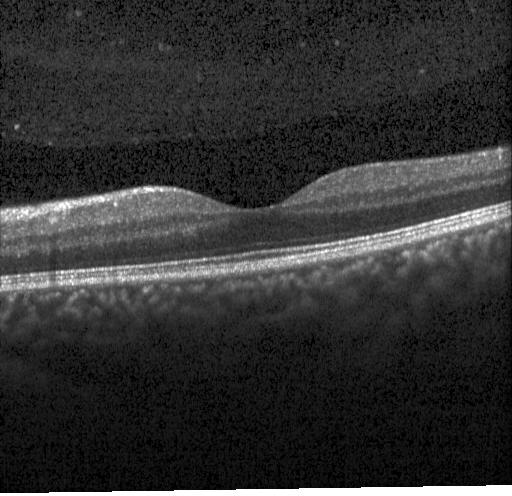

Horizontal scan through the fovea · Heidelberg Spectralis · spectral-domain OCT · optical coherence tomography scan — Finding: no choroidal neovascularization, diabetic macular edema, or drusen.